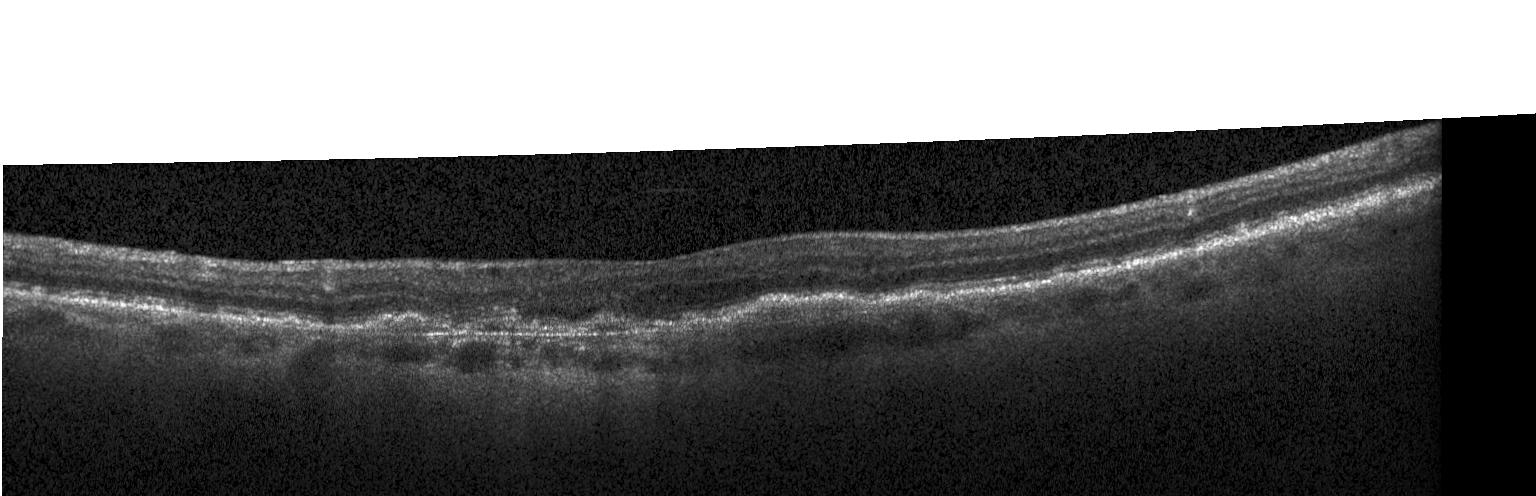

Acquired on a Heidelberg Spectralis · OCT B-scan. This B-scan demonstrates a choroidal neovascular membrane.